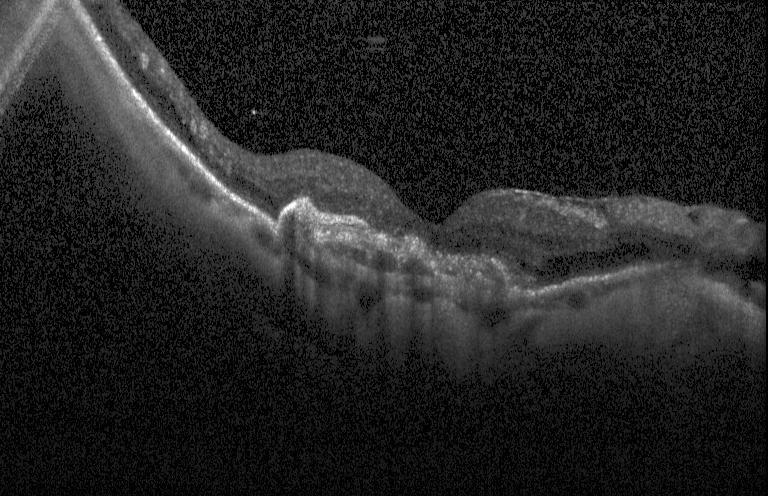

Impression: choroidal neovascularization (CNV).